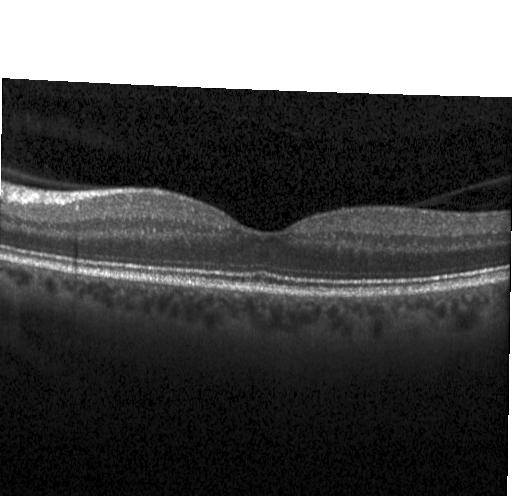

This B-scan demonstrates no evidence of choroidal neovascularization, diabetic macular edema, or drusen.